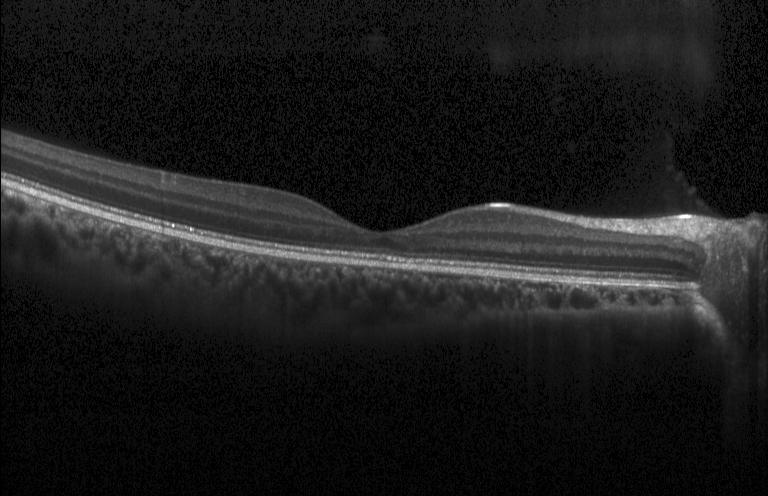

Optical coherence tomography B-scan. Centered on the fovea. Spectral-domain optical coherence tomography
Macular OCT: no CNV, no DME, and no drusen.